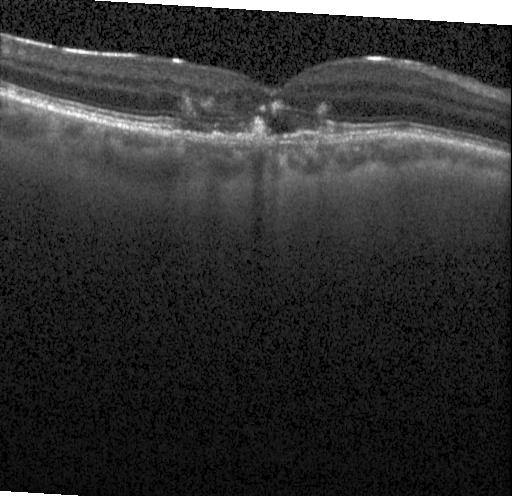

Macular scan · optical coherence tomography B-scan · spectral-domain OCT
Finding: choroidal neovascularization (CNV).